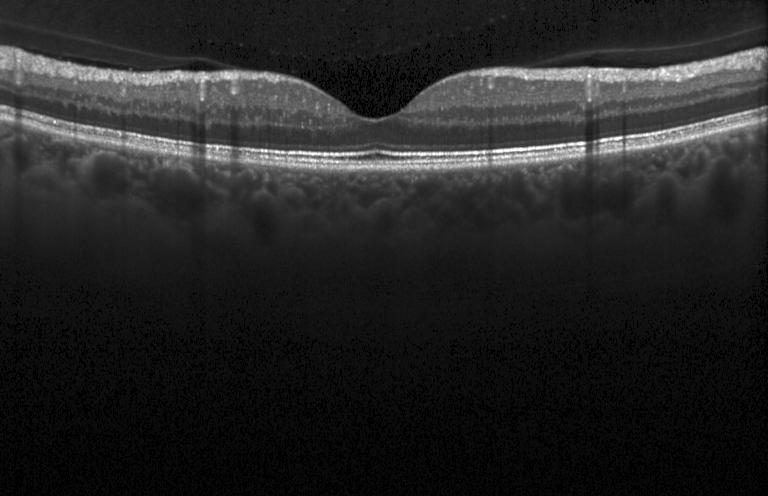 Retinal OCT B-scan, fovea-centered — No CNV, DME, or drusen.